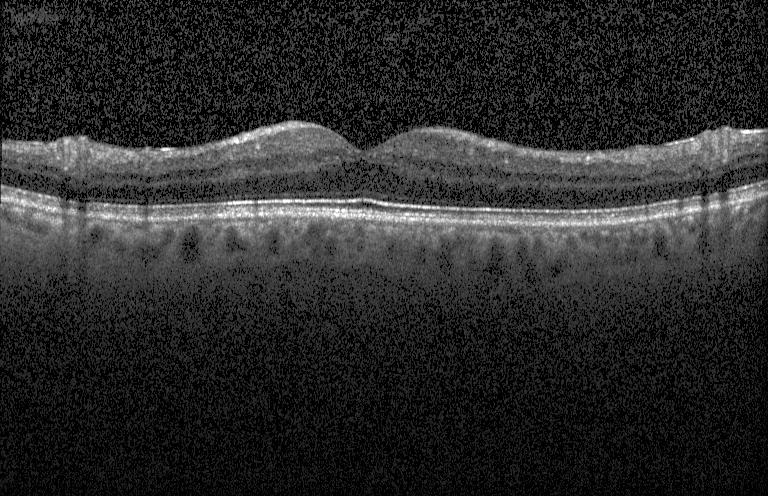
Retinal OCT cross-section showing no evidence of CNV, DME, or drusen.